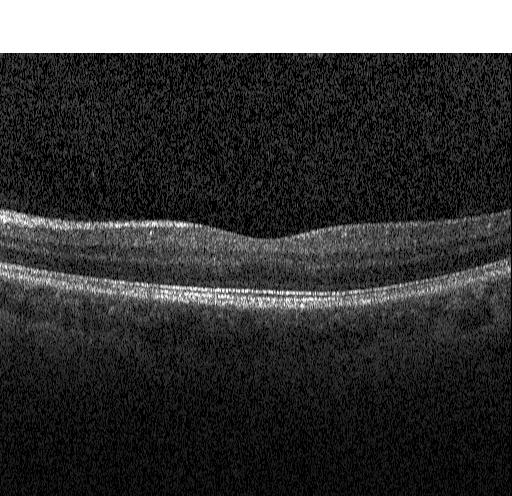

This B-scan demonstrates no choroidal neovascularization, diabetic macular edema, or drusen.